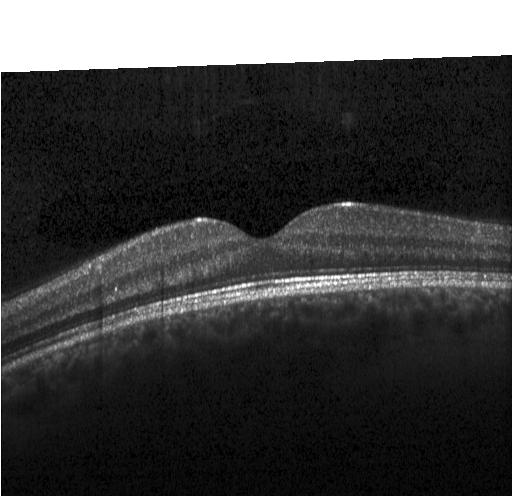
Macular OCT: no choroidal neovascularization, no diabetic macular edema, and no drusen.